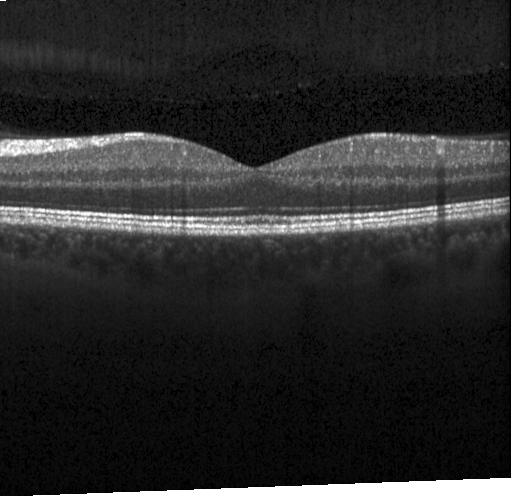 This B-scan demonstrates neither choroidal neovascularization, diabetic macular edema, nor drusen.